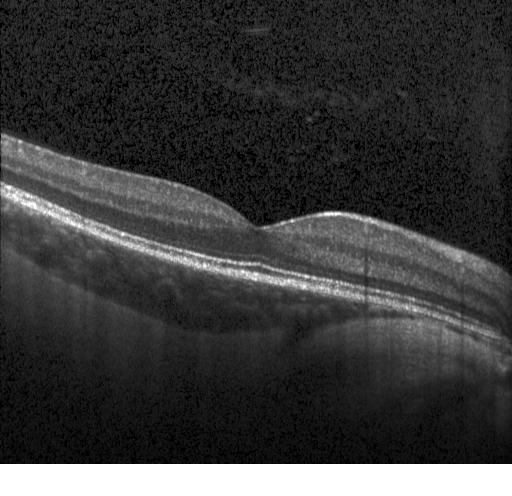
Spectral-domain OCT · optical coherence tomography B-scan · centered on the fovea — Finding: neither choroidal neovascularization, diabetic macular edema, nor drusen.